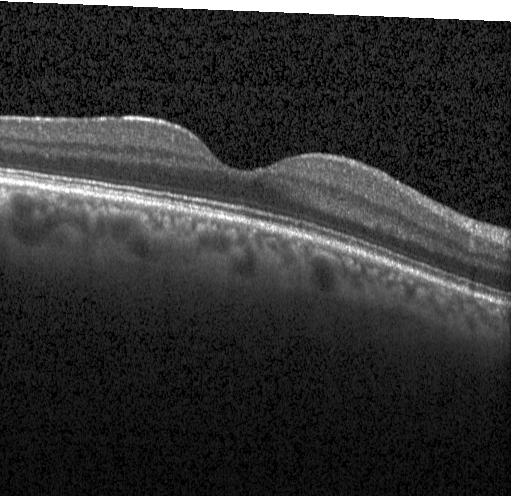

Horizontal scan through the fovea. Optical coherence tomography scan. Spectral-domain OCT. Heidelberg Spectralis — OCT finding: no evidence of CNV, DME, or drusen.